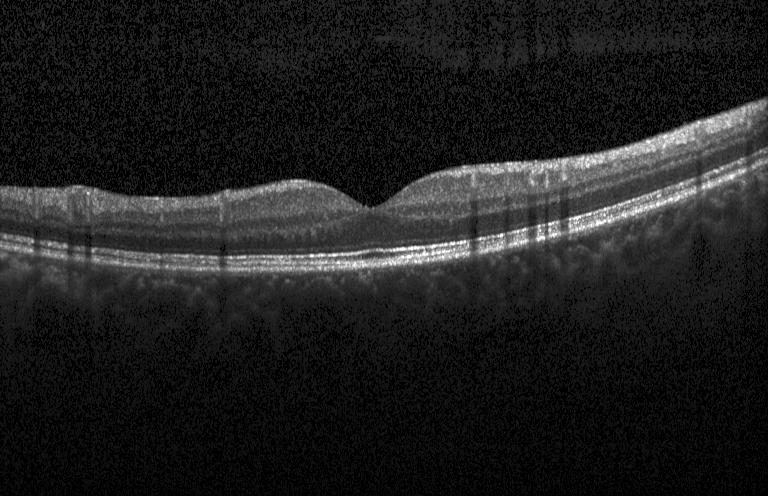 Diagnosis: no choroidal neovascularization, no diabetic macular edema, and no drusen.